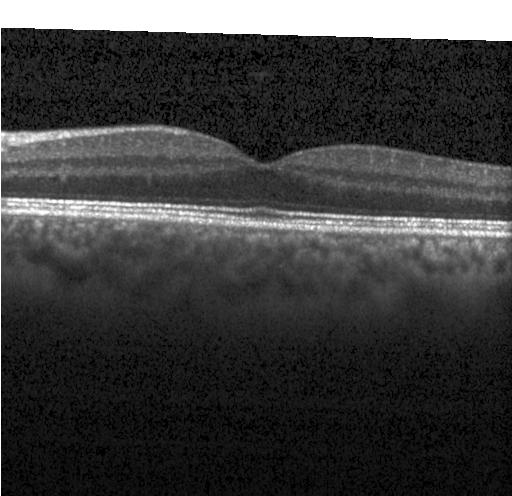

Retinal OCT B-scan, centered on the fovea, spectral-domain OCT. Finding: neither choroidal neovascularization, diabetic macular edema, nor drusen.